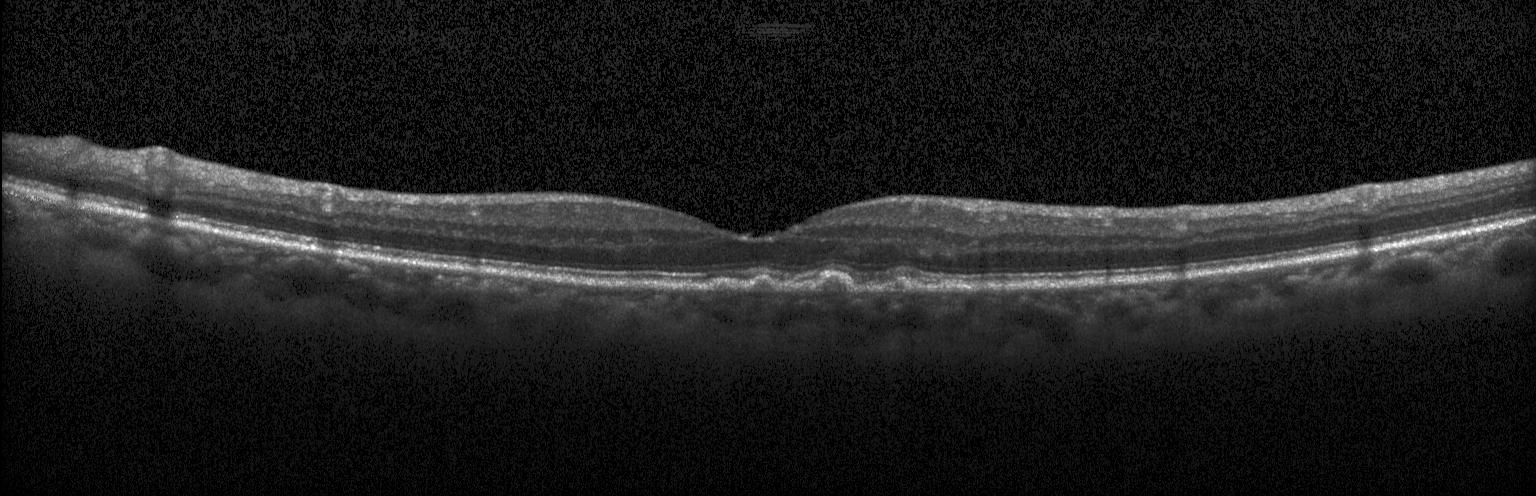 Through the macula; retinal OCT cross-section; spectral-domain optical coherence tomography
Diagnosis: multiple drusen.